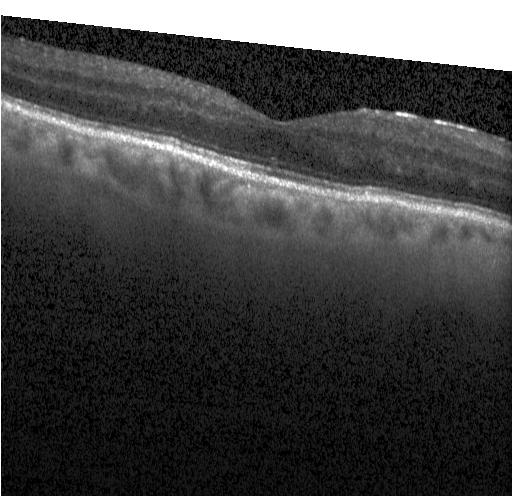
Optical coherence tomography scan. Dx: no choroidal neovascularization, diabetic macular edema, or drusen.